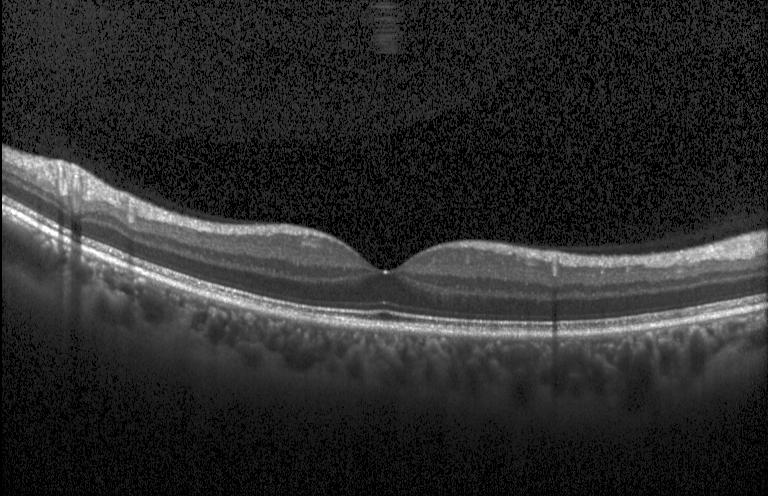 Optical coherence tomography scan, spectral-domain OCT, acquired on a Heidelberg Spectralis, fovea-centered — Finding: no evidence of choroidal neovascularization, diabetic macular edema, or drusen.